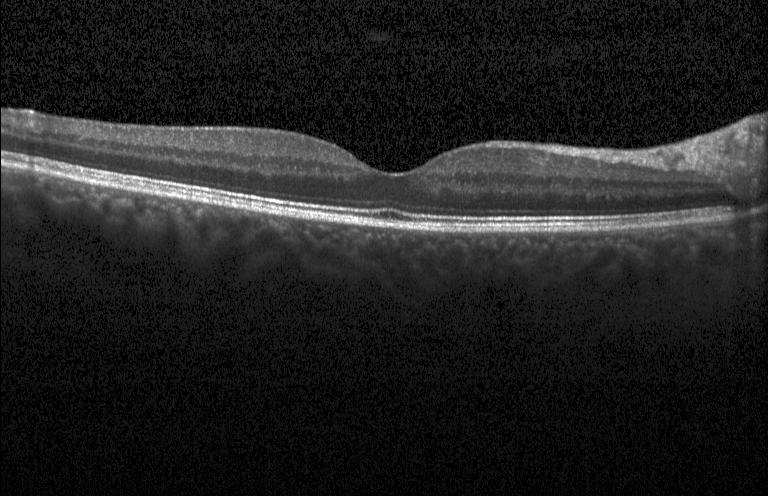
OCT B-scan · macular scan — Impression: no evidence of CNV, DME, or drusen.